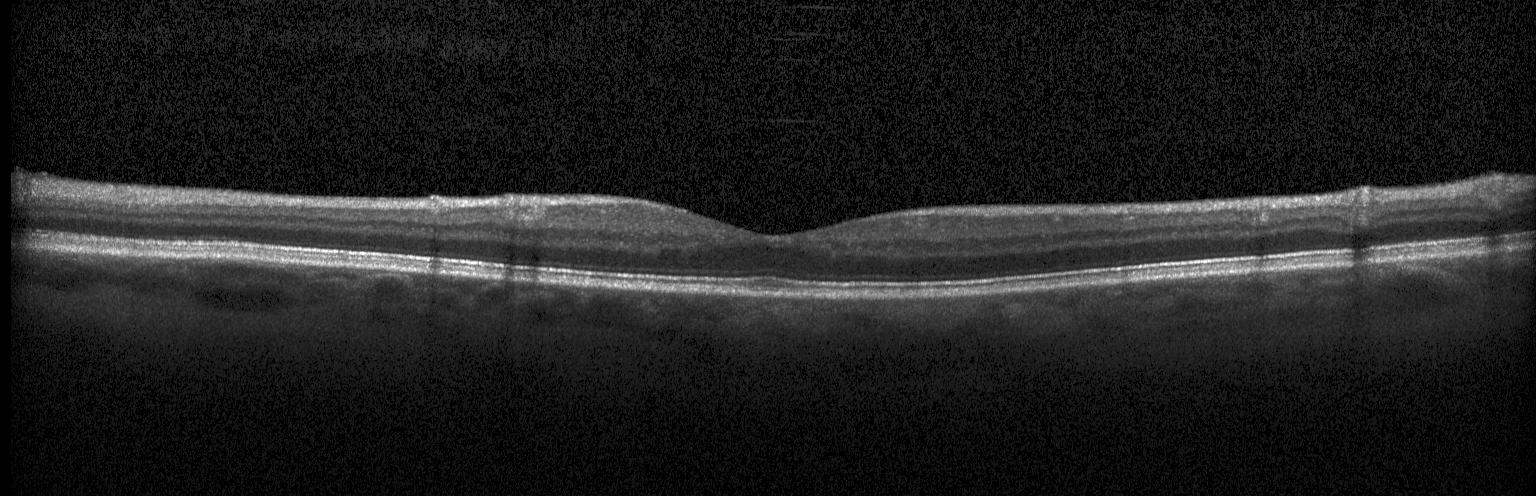 Spectral-domain OCT; Heidelberg Spectralis; OCT B-scan; centered on the fovea. Finding: no choroidal neovascularization, diabetic macular edema, or drusen.